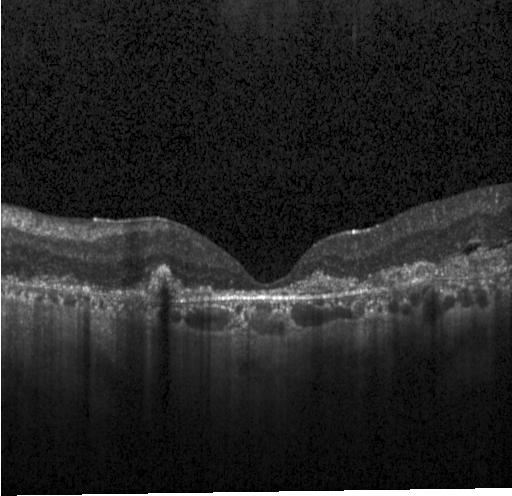 Retinal OCT cross-section · horizontal scan through the fovea
Dx: a choroidal neovascular membrane.